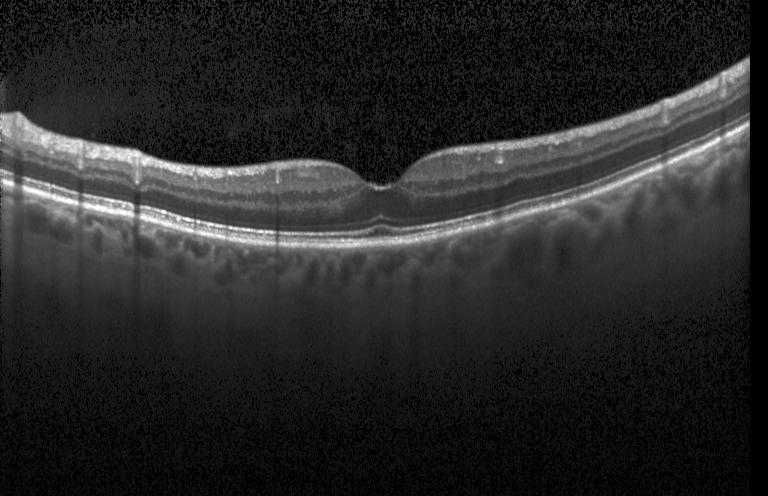
Impression: no choroidal neovascularization, diabetic macular edema, or drusen.